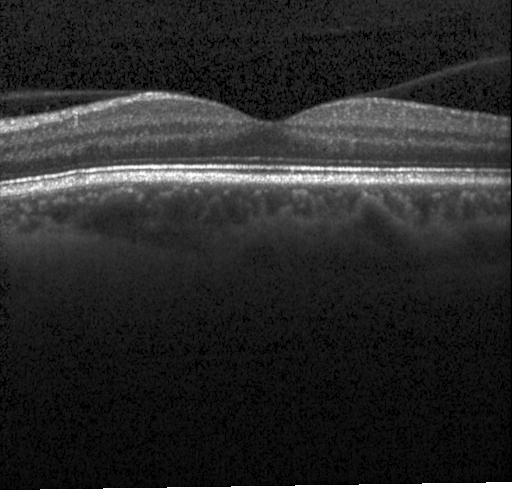
This B-scan demonstrates no evidence of CNV, DME, or drusen.